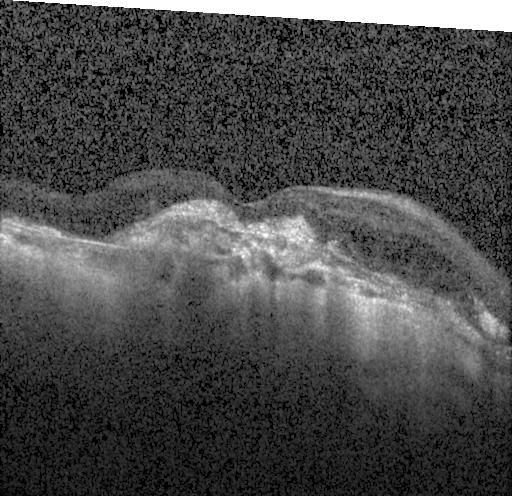

SD-OCT, instrument: Heidelberg Spectralis, optical coherence tomography scan.
OCT finding: a choroidal neovascular membrane.